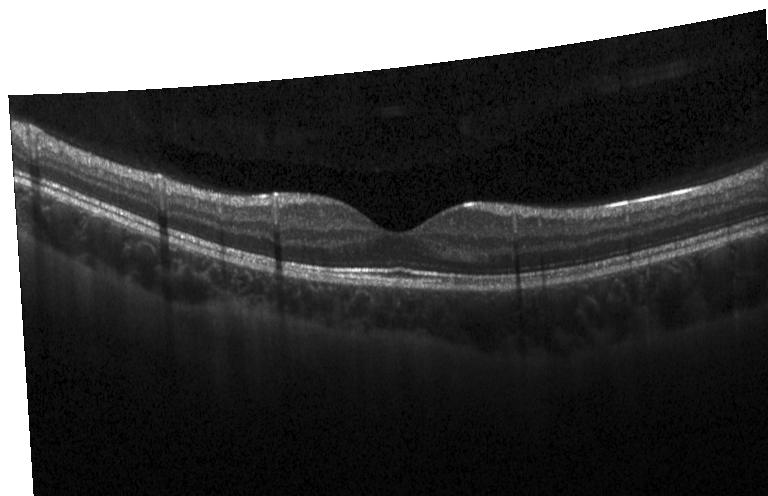

Dx: neither choroidal neovascularization, diabetic macular edema, nor drusen.